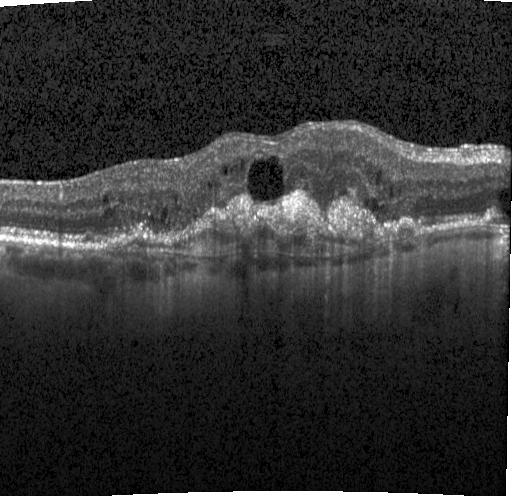
Acquired on a Heidelberg Spectralis, spectral-domain OCT, OCT line scan. Assessment: choroidal neovascularization (CNV).